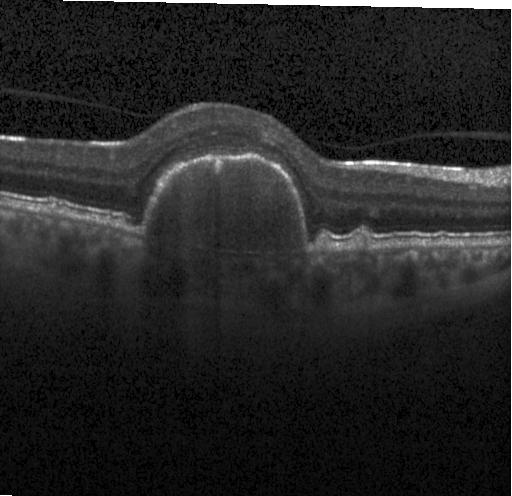

Diagnosis: a choroidal neovascular membrane.